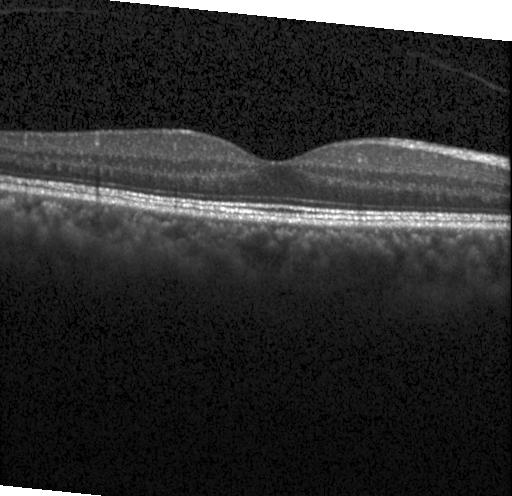 OCT finding: no CNV, no DME, and no drusen.